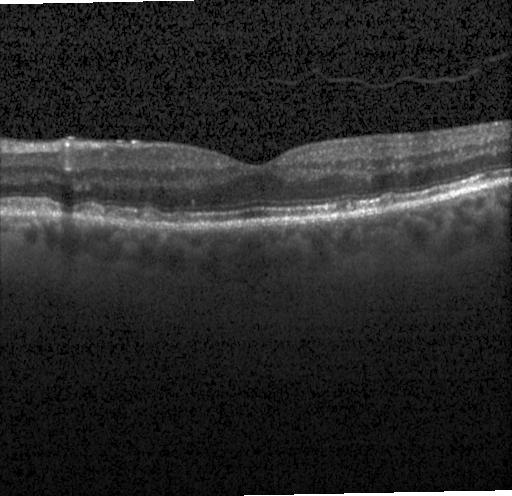
Acquired on a Heidelberg Spectralis. OCT line scan. SD-OCT
Impression: sub-RPE drusenoid deposits.